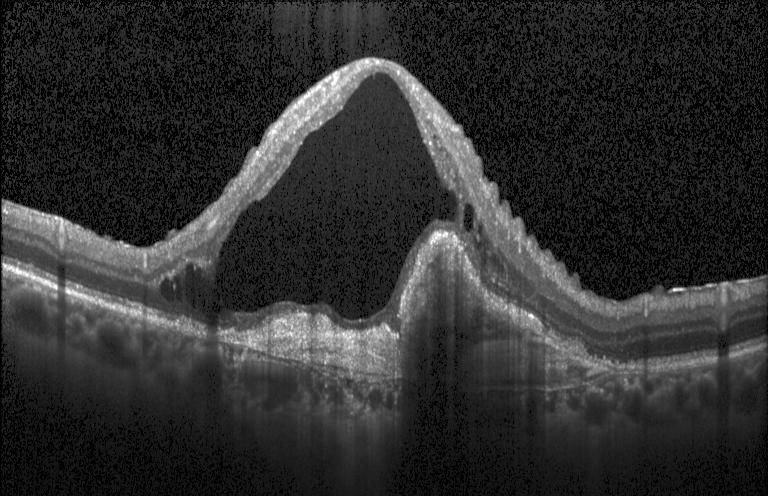 Spectral-domain optical coherence tomography, OCT B-scan, instrument: Heidelberg Spectralis. Impression: choroidal neovascularization (CNV).